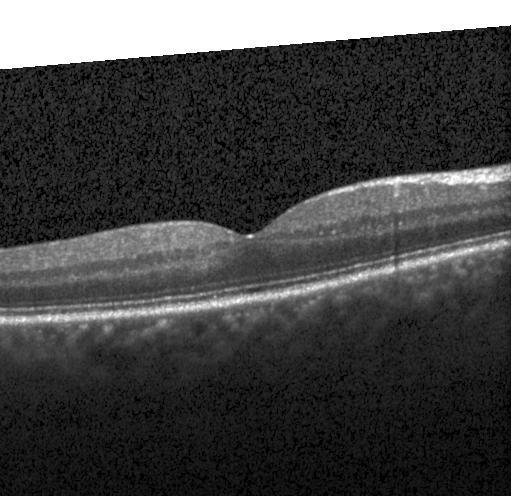

Spectral-domain OCT. OCT B-scan. Centered on the fovea
Finding: no CNV, no DME, and no drusen.